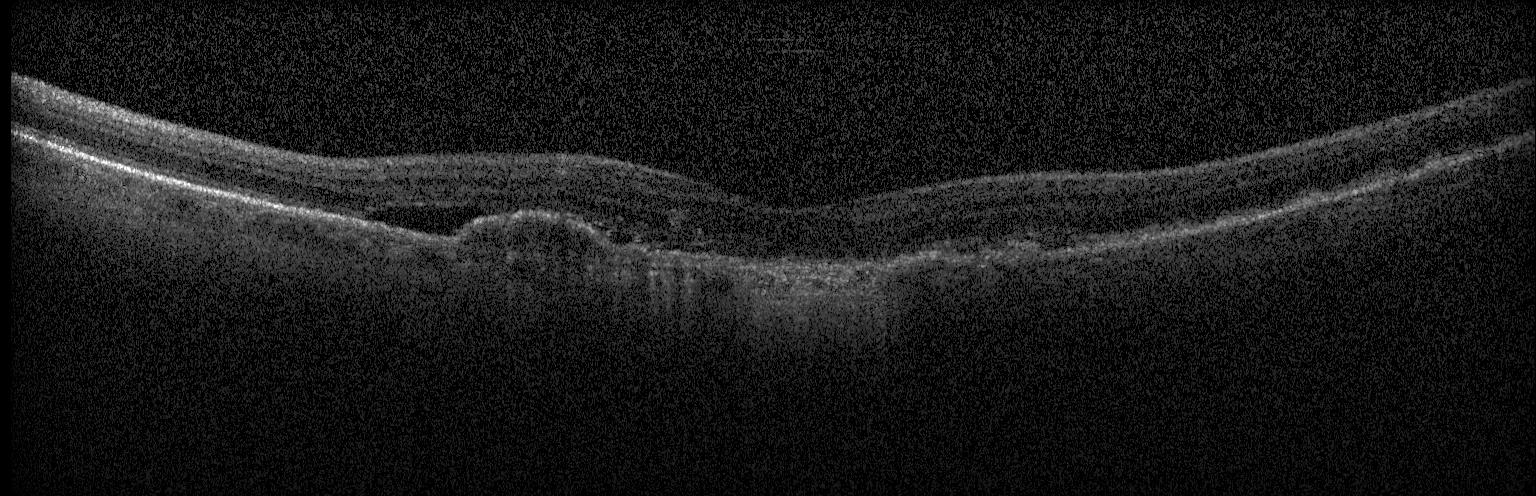
Optical coherence tomography scan, acquired on a Heidelberg Spectralis, SD-OCT.
This B-scan demonstrates a choroidal neovascular membrane.